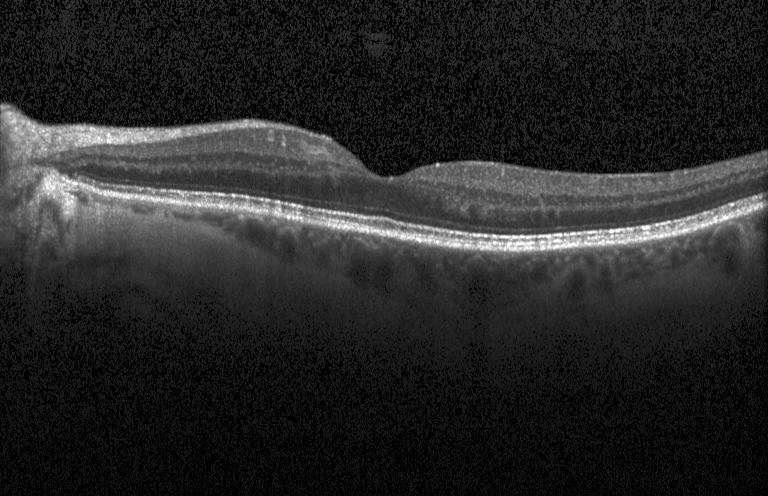 Heidelberg Spectralis OCT system. Spectral-domain optical coherence tomography. OCT B-scan
Dx: no choroidal neovascularization, no diabetic macular edema, and no drusen.